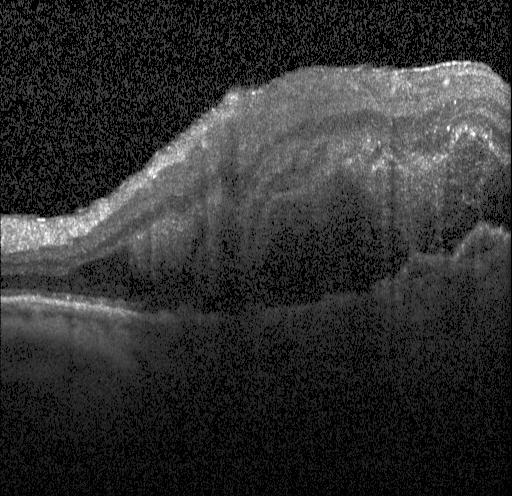
Diagnosis: choroidal neovascularization (CNV).